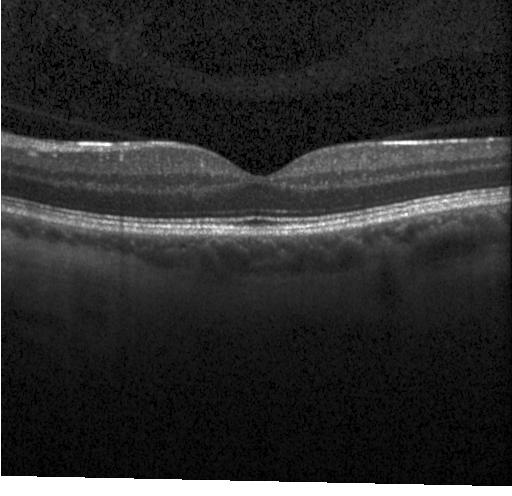
Impression: no evidence of choroidal neovascularization, diabetic macular edema, or drusen.